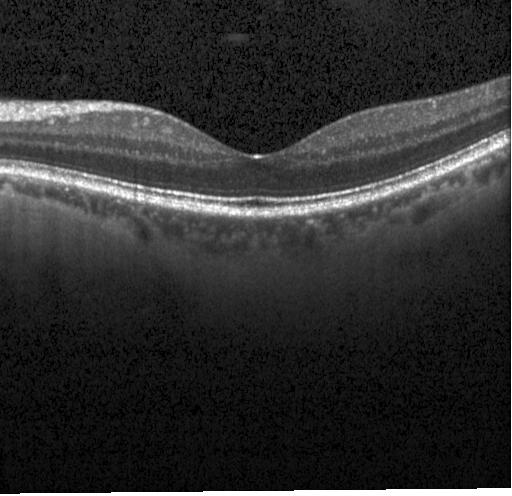
Heidelberg Spectralis OCT system; centered on the fovea; optical coherence tomography scan; spectral-domain optical coherence tomography. Assessment: neither choroidal neovascularization, diabetic macular edema, nor drusen.